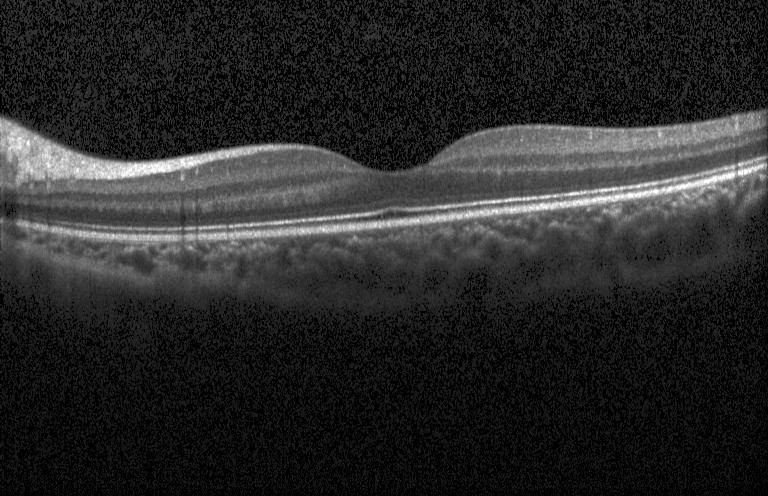 Diagnosis: no CNV, DME, or drusen.